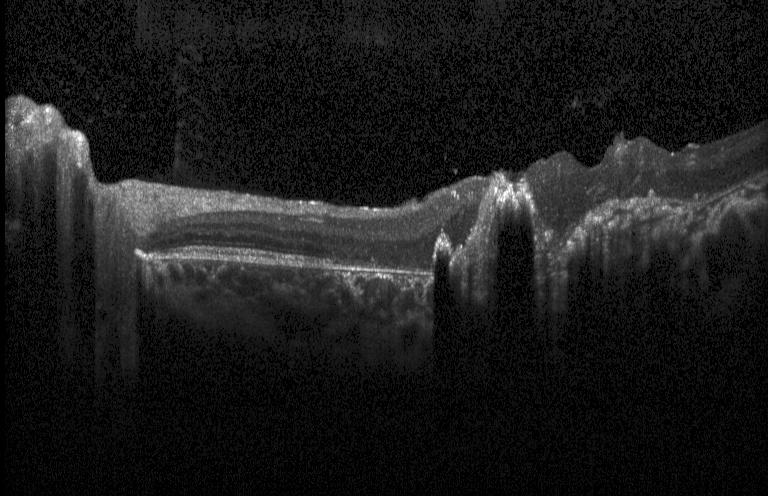
Macular OCT: CNV.